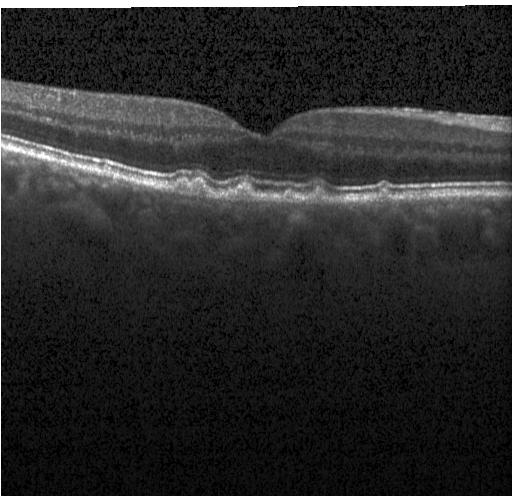

Diagnosis: multiple drusen.